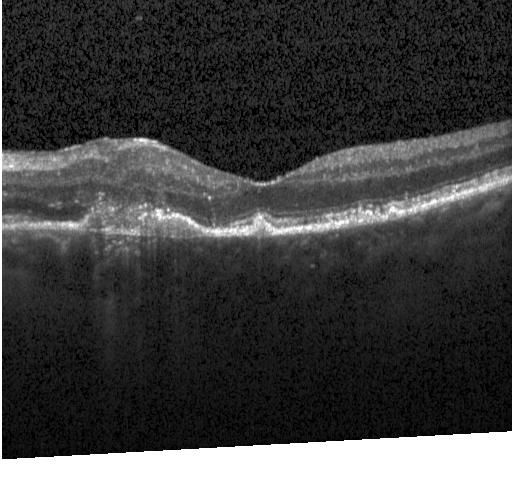 Impression: CNV.